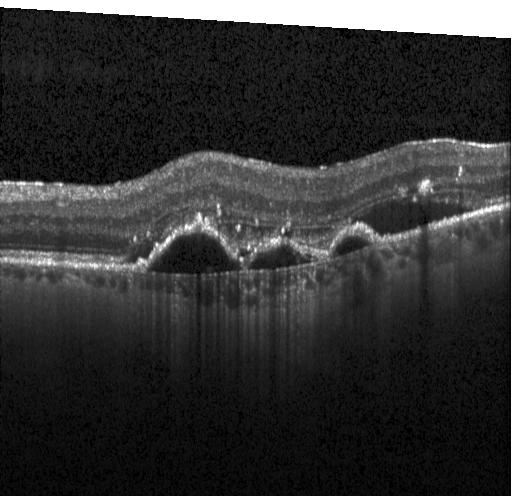 Impression: choroidal neovascularization.